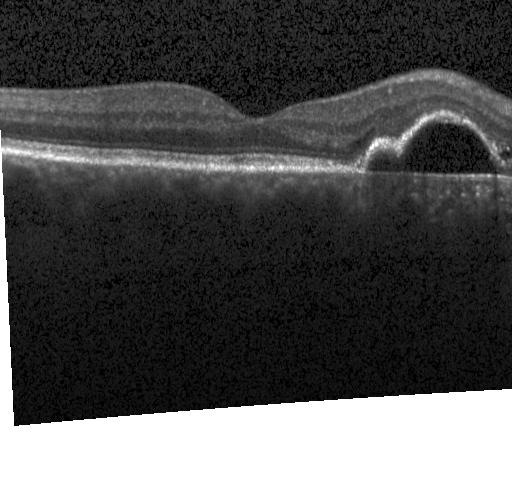

Optical coherence tomography scan.
Diagnosis: CNV.